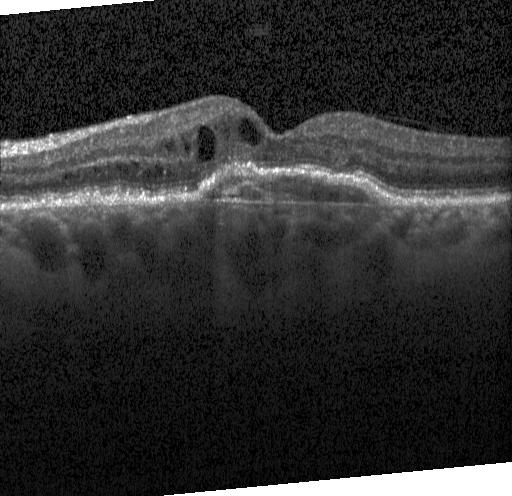

OCT B-scan, spectral-domain optical coherence tomography, acquired on a Heidelberg Spectralis
Impression: a choroidal neovascular membrane.